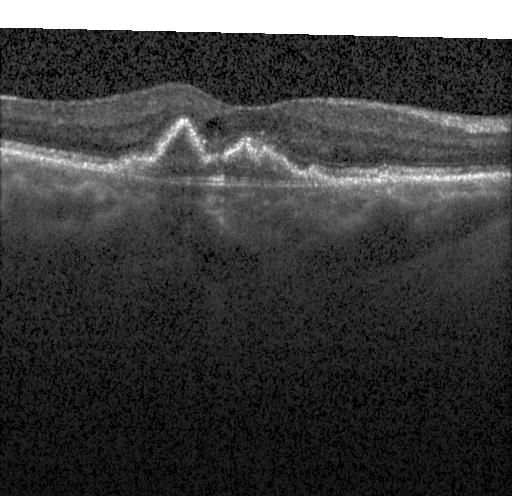

Diagnosis: CNV.